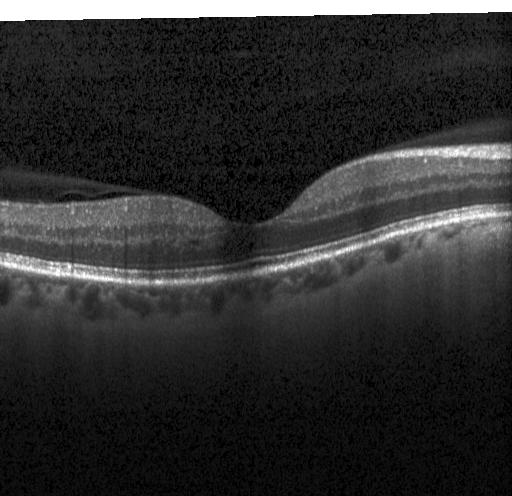

Finding: no choroidal neovascularization, diabetic macular edema, or drusen.